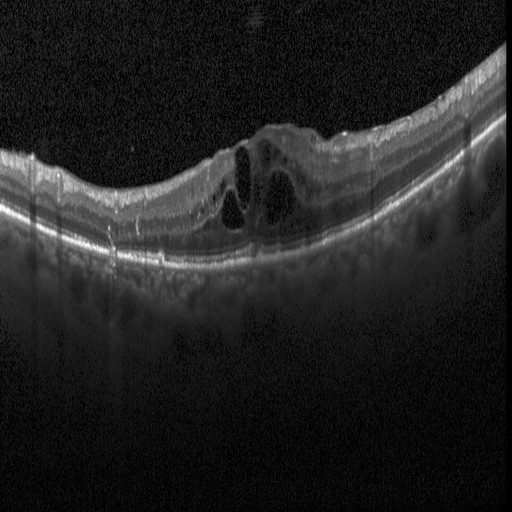

Centered on the fovea, Heidelberg Spectralis OCT system, spectral-domain optical coherence tomography, OCT line scan — This B-scan demonstrates diabetic macular edema.